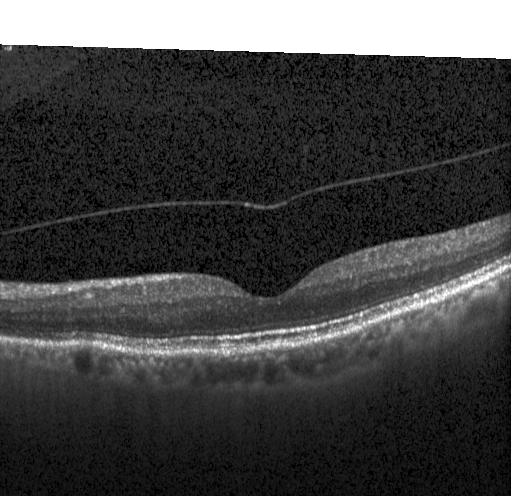
No choroidal neovascularization, no diabetic macular edema, and no drusen.